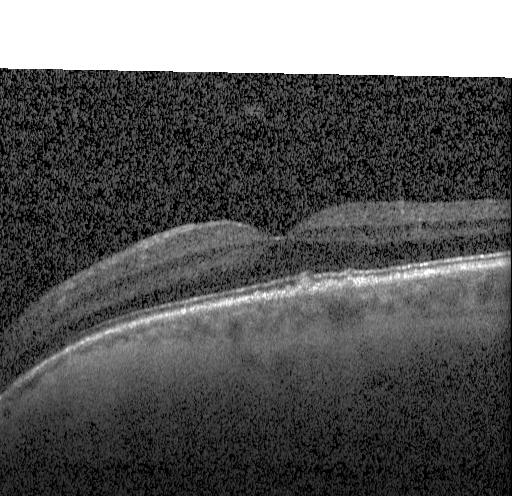
Optical coherence tomography B-scan; macular scan; spectral-domain OCT; acquired on a Heidelberg Spectralis. Macular OCT: multiple drusen.